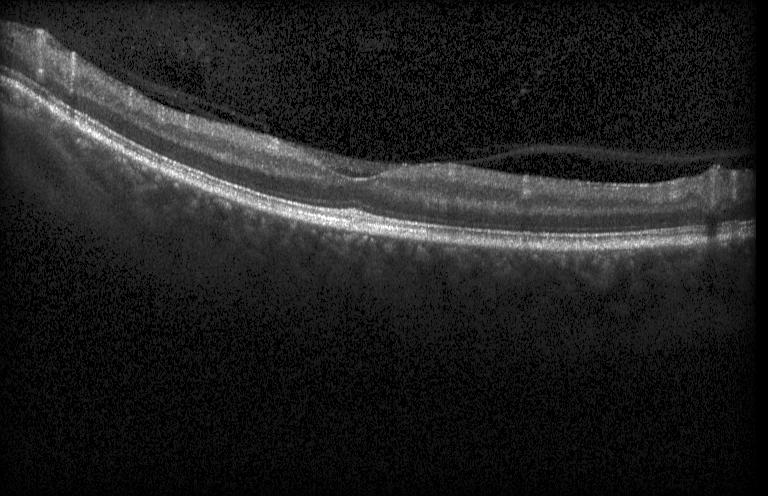

Acquired on a Heidelberg Spectralis. Horizontal scan through the fovea. Spectral-domain OCT. Optical coherence tomography B-scan.
Finding: no choroidal neovascularization, no diabetic macular edema, and no drusen.